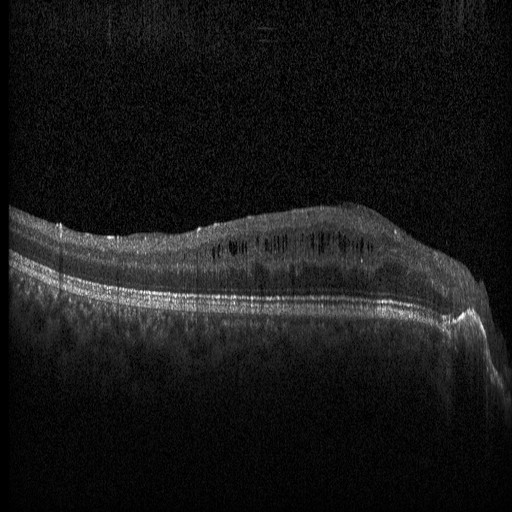

SD-OCT; horizontal scan through the fovea; optical coherence tomography B-scan — Diagnosis: diabetic macular edema.